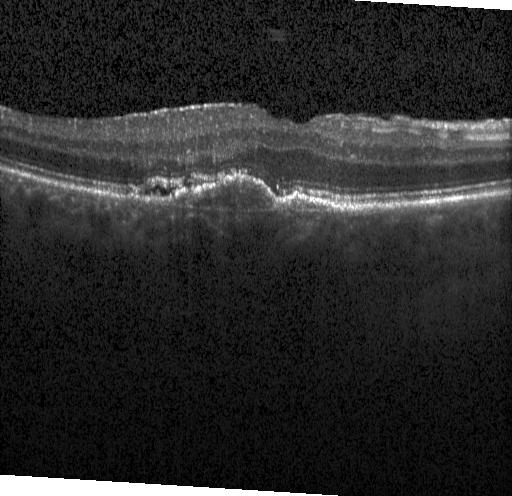 Optical coherence tomography scan, spectral-domain OCT, Heidelberg Spectralis OCT system.
The scan shows a choroidal neovascular membrane.